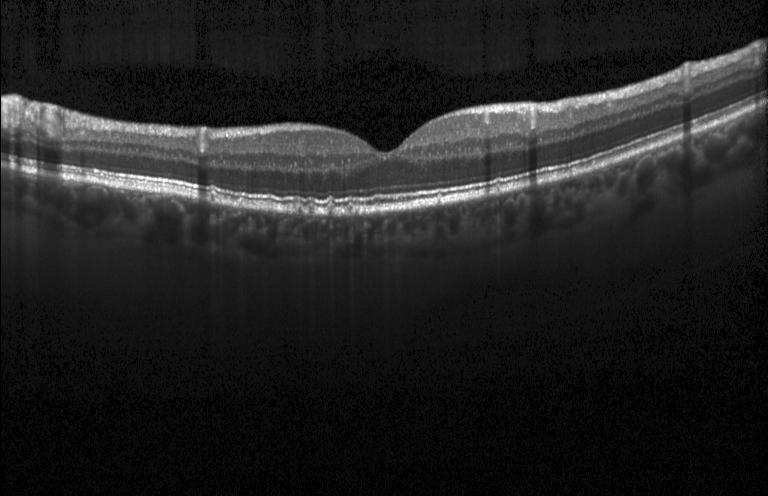
Finding: sub-RPE drusenoid deposits.